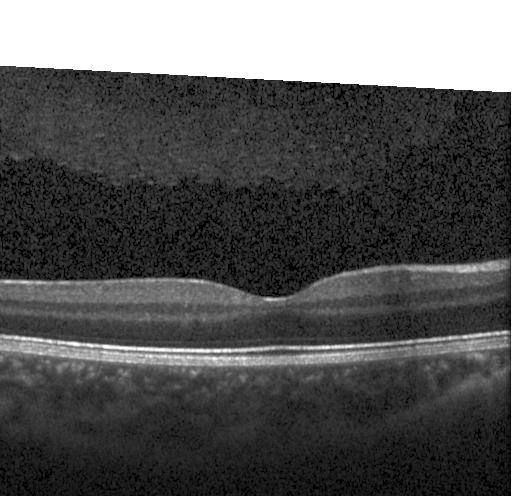

Optical coherence tomography scan · SD-OCT. Diagnosis: no evidence of CNV, DME, or drusen.